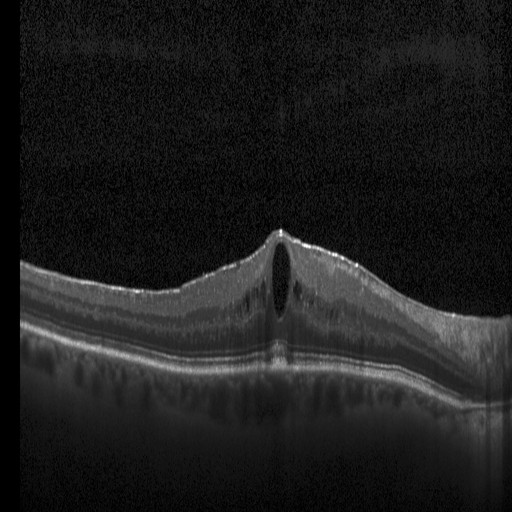 Retinal OCT B-scan; centered on the fovea; instrument: Heidelberg Spectralis; spectral-domain optical coherence tomography
DME.